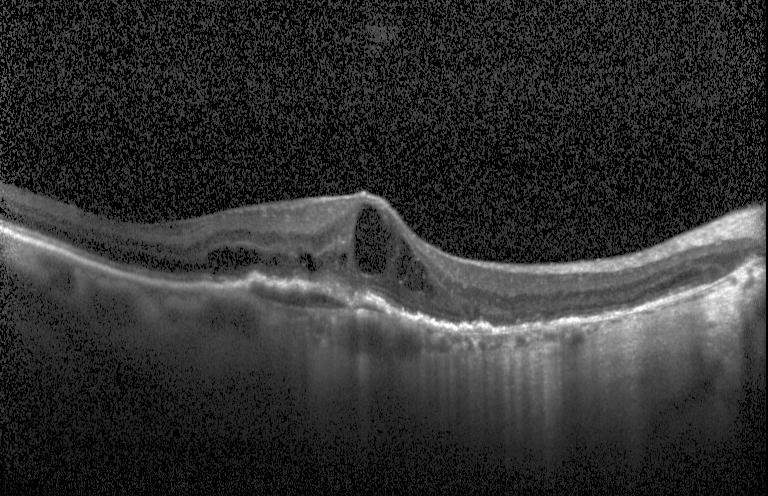 Retinal OCT cross-section; Heidelberg Spectralis OCT system; horizontal scan through the fovea
Finding: a choroidal neovascular membrane.